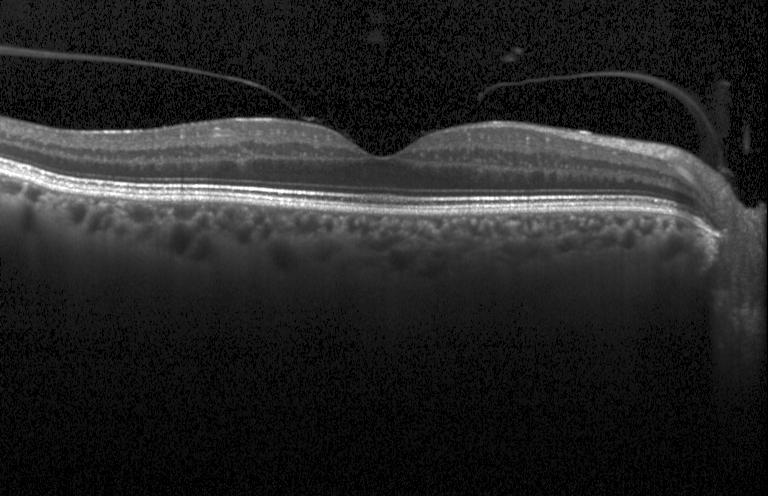
Optical coherence tomography scan, spectral-domain optical coherence tomography. Neither choroidal neovascularization, diabetic macular edema, nor drusen.